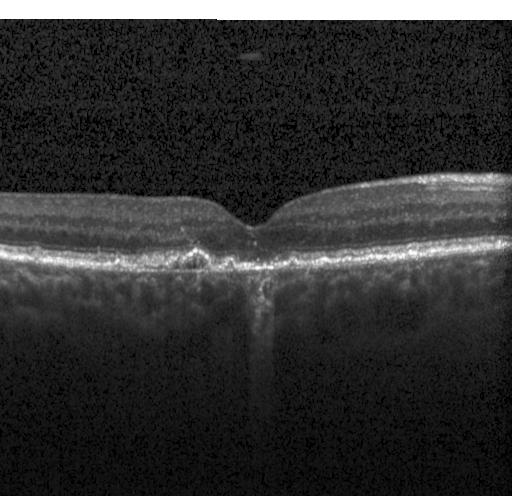

Finding: a choroidal neovascular membrane.